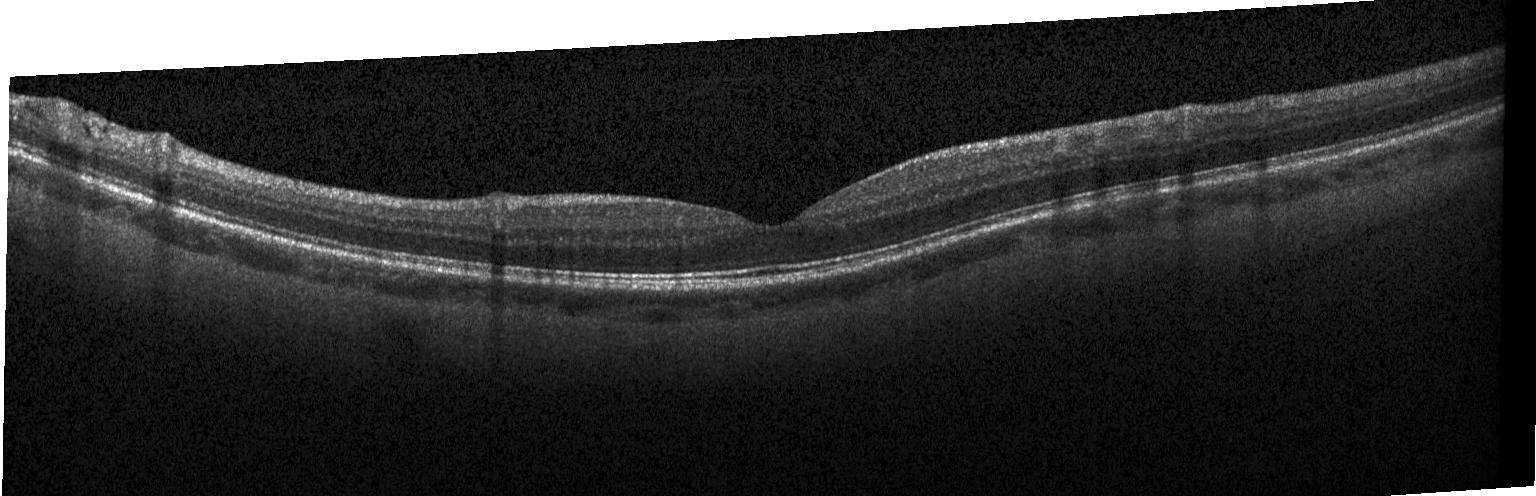 Centered on the fovea. Spectral-domain optical coherence tomography. Optical coherence tomography B-scan. Heidelberg Spectralis. Finding: neither choroidal neovascularization, diabetic macular edema, nor drusen.